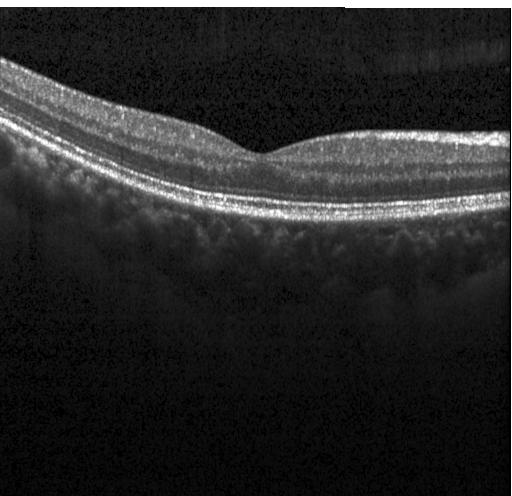
Optical coherence tomography B-scan. Spectral-domain optical coherence tomography. Centered on the fovea. Heidelberg Spectralis OCT system. Impression: no CNV, no DME, and no drusen.